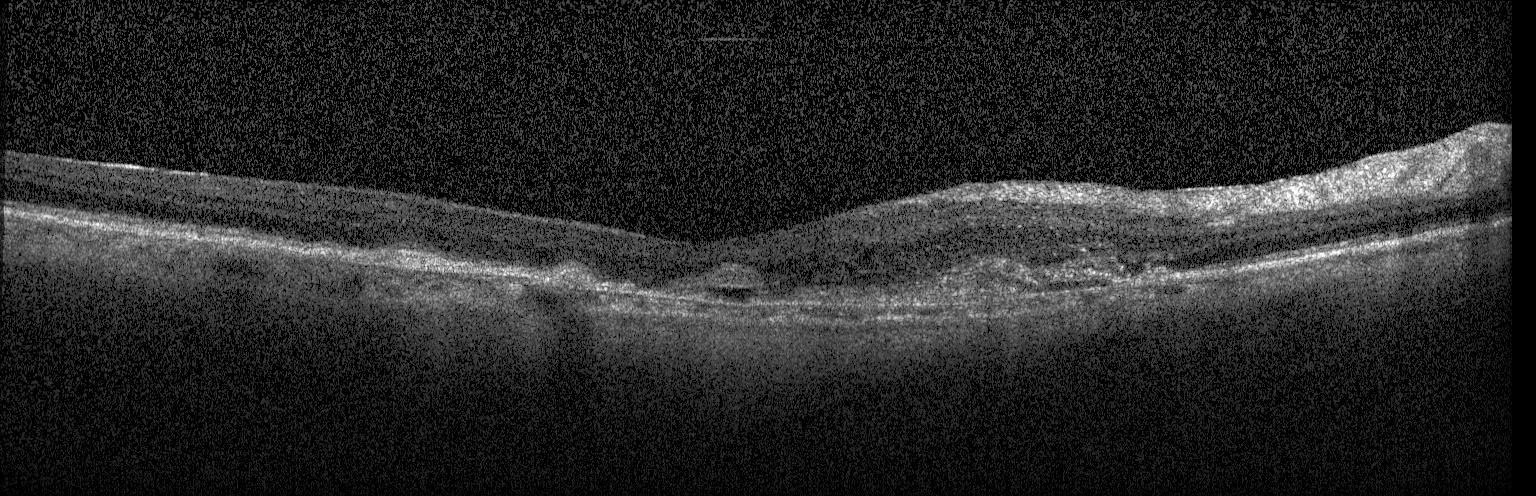

Horizontal scan through the fovea · retinal OCT B-scan · spectral-domain OCT.
The scan shows choroidal neovascularization (CNV).